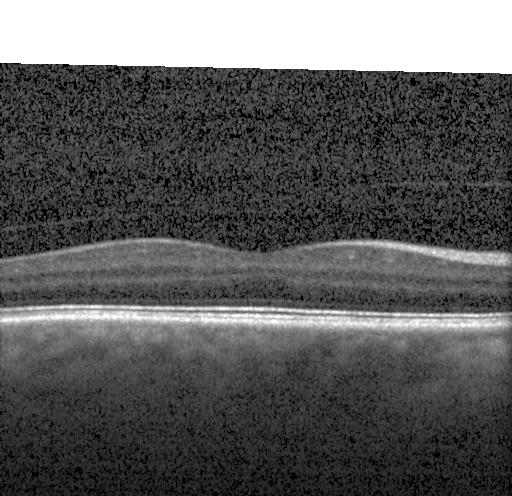
Retinal OCT B-scan
Diagnosis: neither choroidal neovascularization, diabetic macular edema, nor drusen.